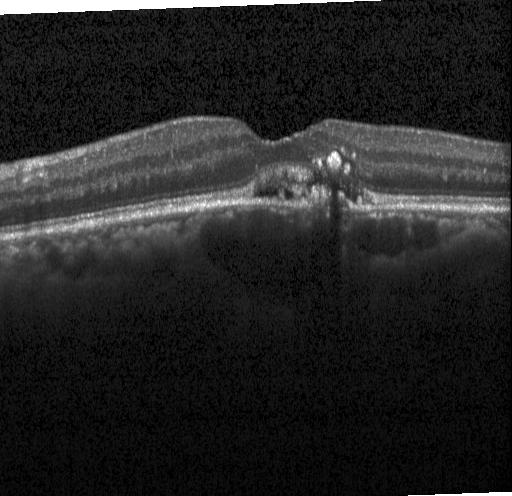 Finding: CNV.